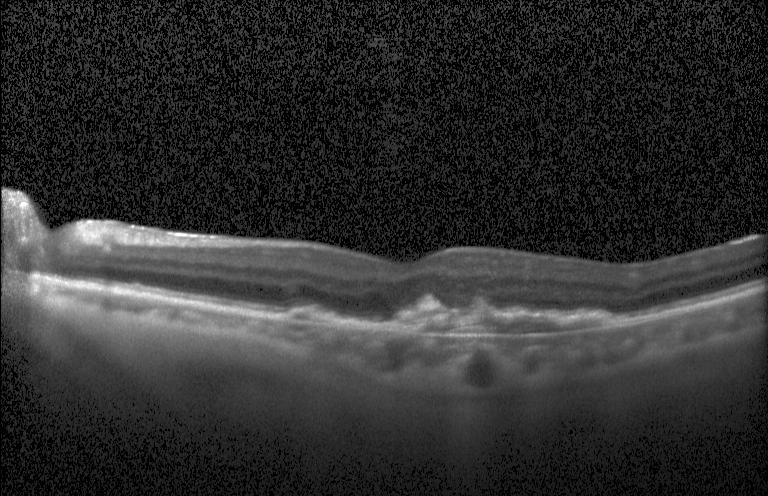 Optical coherence tomography scan; SD-OCT; through the macula; Heidelberg Spectralis OCT system.
Dx: choroidal neovascularization (CNV).